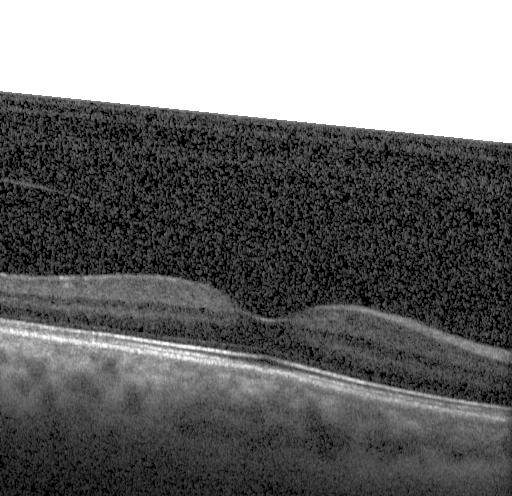
Spectral-domain OCT · acquired on a Heidelberg Spectralis · centered on the fovea · retinal OCT B-scan. Macular OCT: no choroidal neovascularization, no diabetic macular edema, and no drusen.